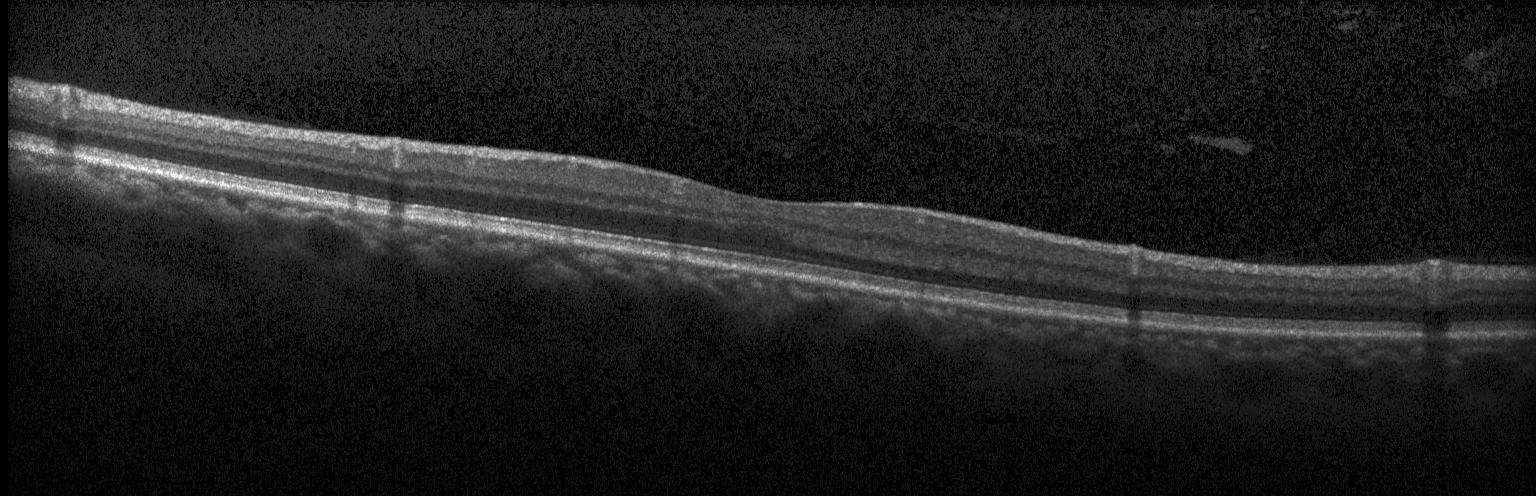

Spectral-domain OCT. Retinal OCT cross-section. Instrument: Heidelberg Spectralis
Assessment: no choroidal neovascularization, diabetic macular edema, or drusen.